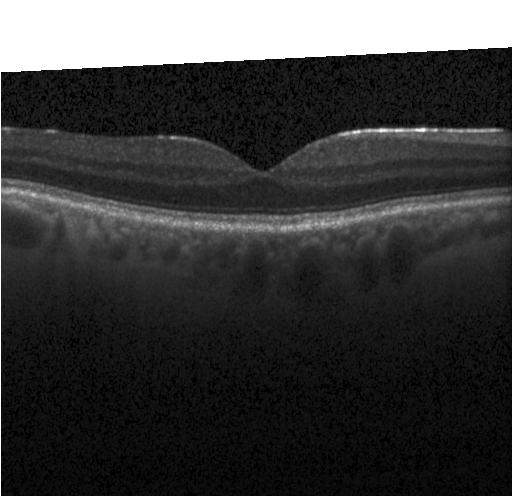 OCT finding: no evidence of choroidal neovascularization, diabetic macular edema, or drusen.